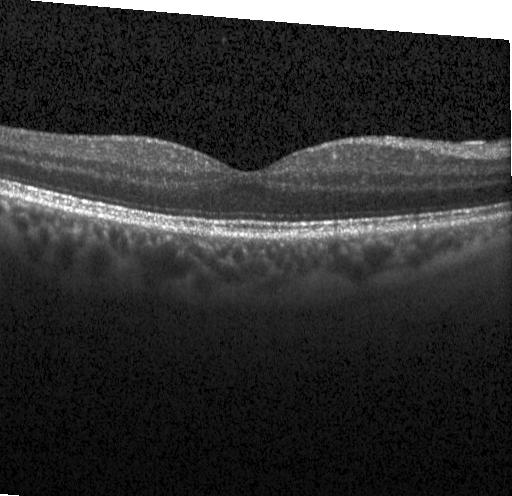 Through the macula; spectral-domain OCT; OCT B-scan; acquired on a Heidelberg Spectralis. The scan shows neither choroidal neovascularization, diabetic macular edema, nor drusen.